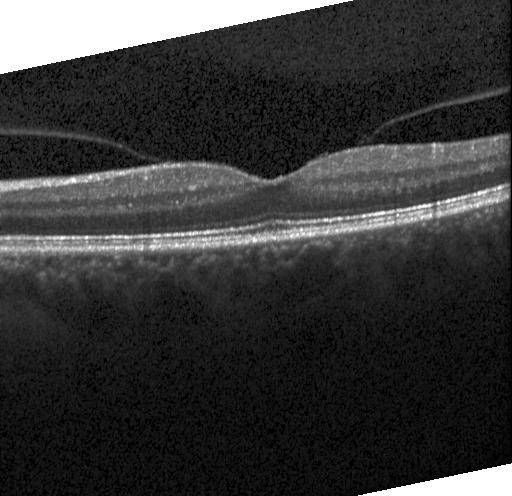

Optical coherence tomography B-scan, horizontal scan through the fovea, acquired on a Heidelberg Spectralis, spectral-domain optical coherence tomography
This B-scan demonstrates no evidence of CNV, DME, or drusen.